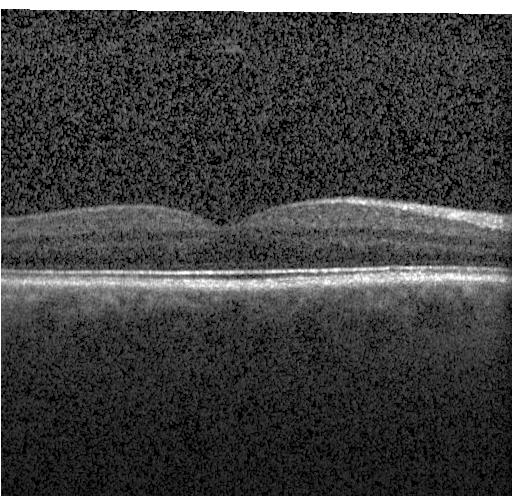 Assessment: no CNV, DME, or drusen.